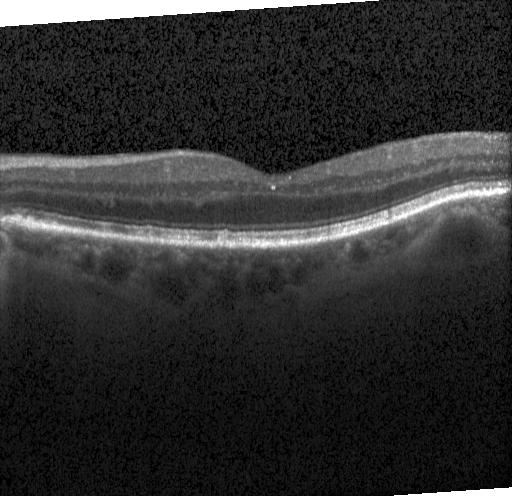
Optical coherence tomography scan. This B-scan demonstrates sub-RPE drusenoid deposits.